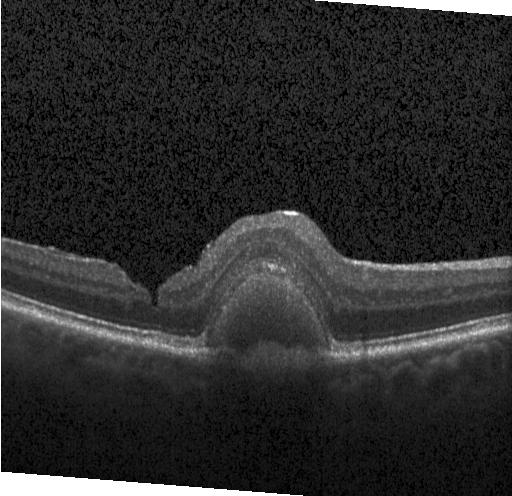

OCT B-scan showing choroidal neovascularization.